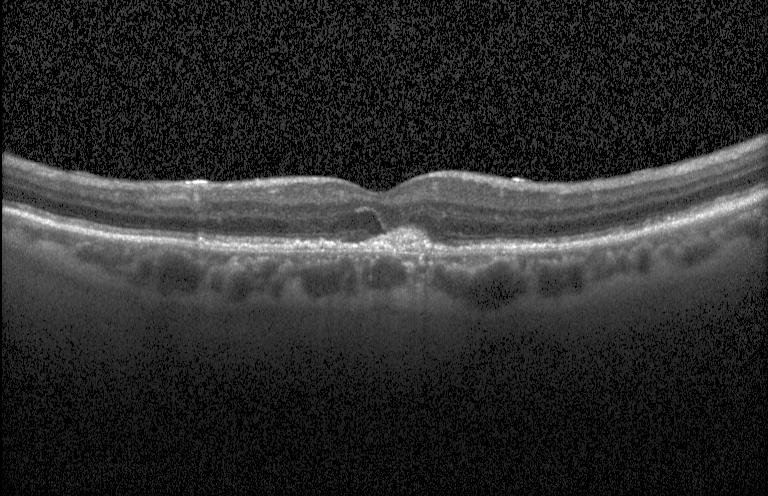

Retinal OCT B-scan — Assessment: a choroidal neovascular membrane.